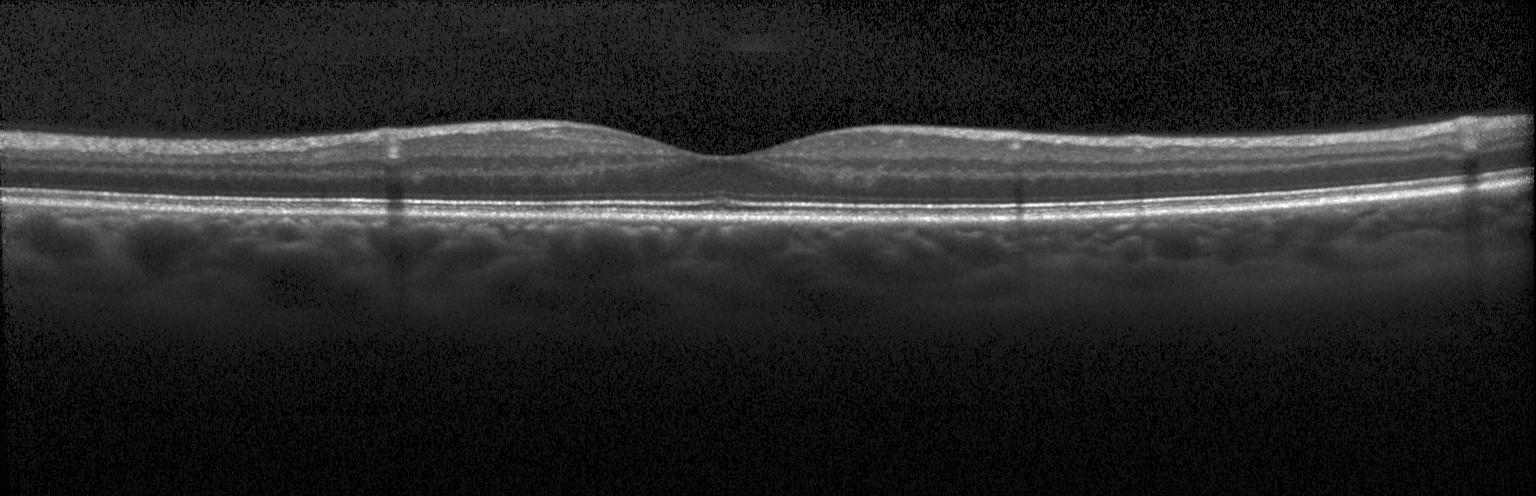 OCT B-scan. SD-OCT. Heidelberg Spectralis.
This B-scan demonstrates no choroidal neovascularization, diabetic macular edema, or drusen.